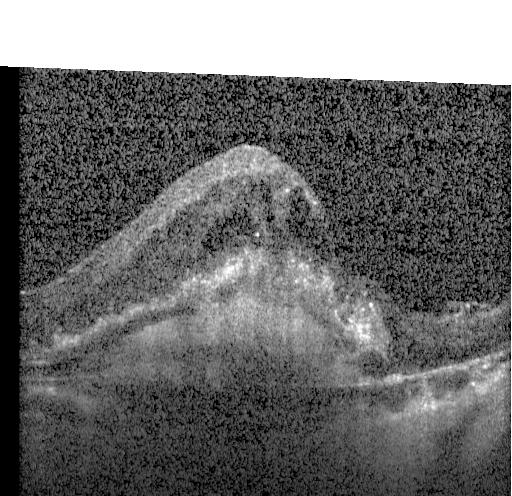
Diagnosis: a choroidal neovascular membrane.